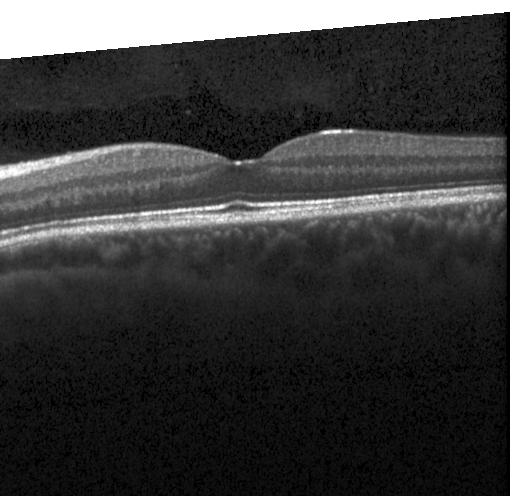

Macular OCT: neither CNV, DME, nor drusen.